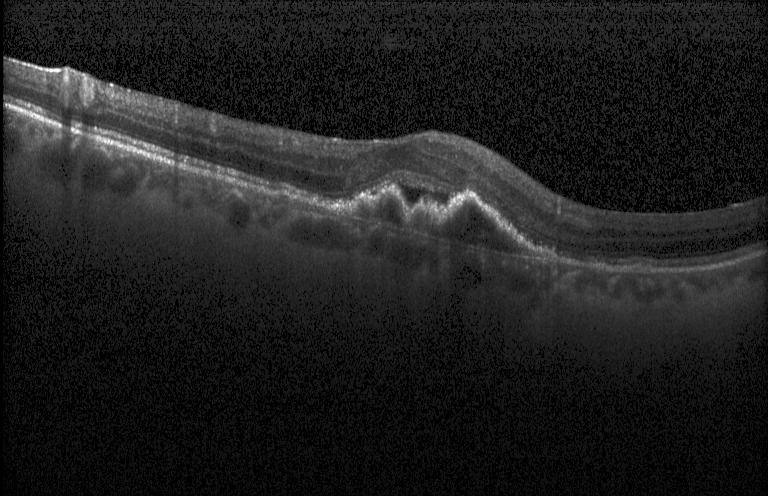 Macular OCT demonstrating CNV.